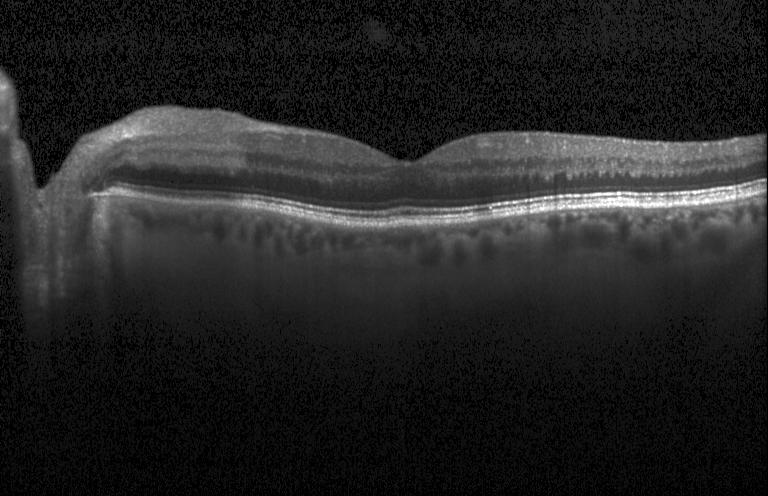
Fovea-centered; retinal OCT cross-section; SD-OCT; Heidelberg Spectralis. The scan shows no evidence of choroidal neovascularization, diabetic macular edema, or drusen.